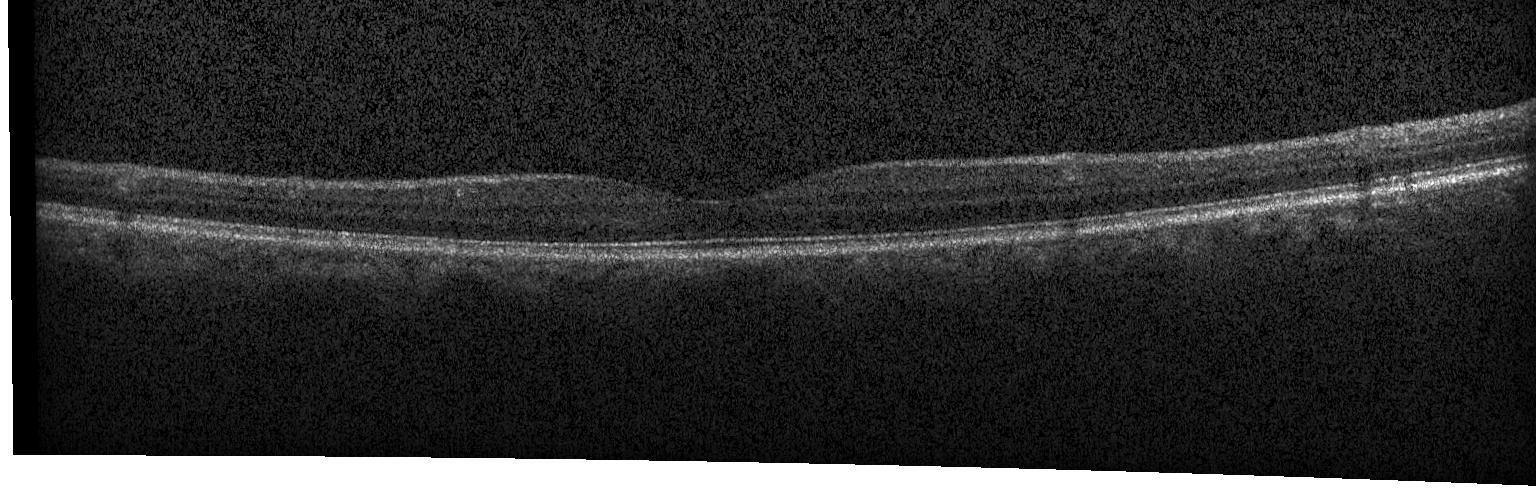

Diagnosis: no evidence of CNV, DME, or drusen.